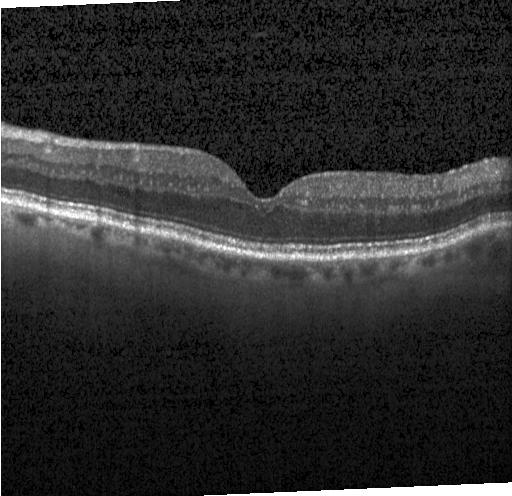
Macular OCT: neither choroidal neovascularization, diabetic macular edema, nor drusen.